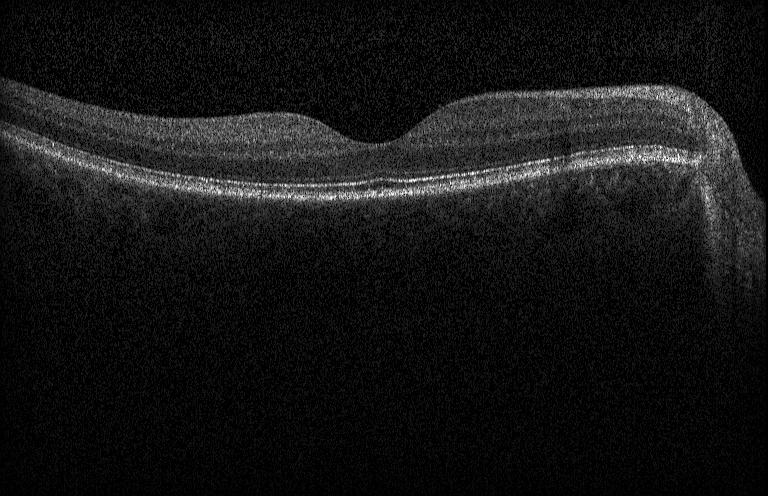
OCT finding: neither choroidal neovascularization, diabetic macular edema, nor drusen.